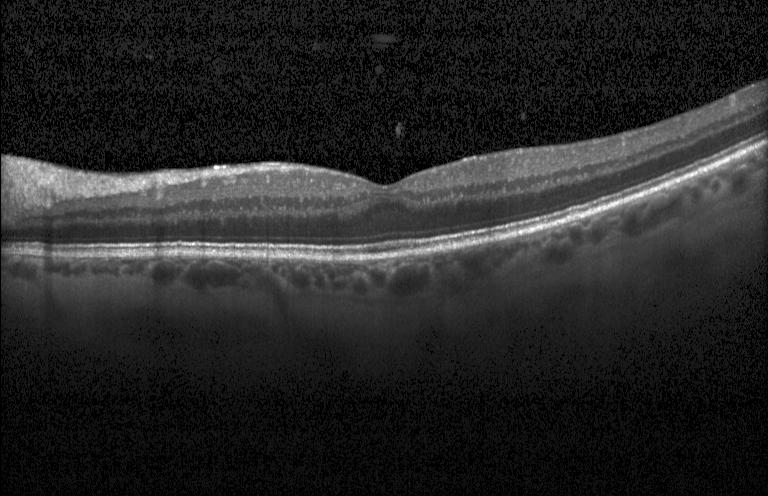
Optical coherence tomography scan; macular scan.
Assessment: no CNV, no DME, and no drusen.